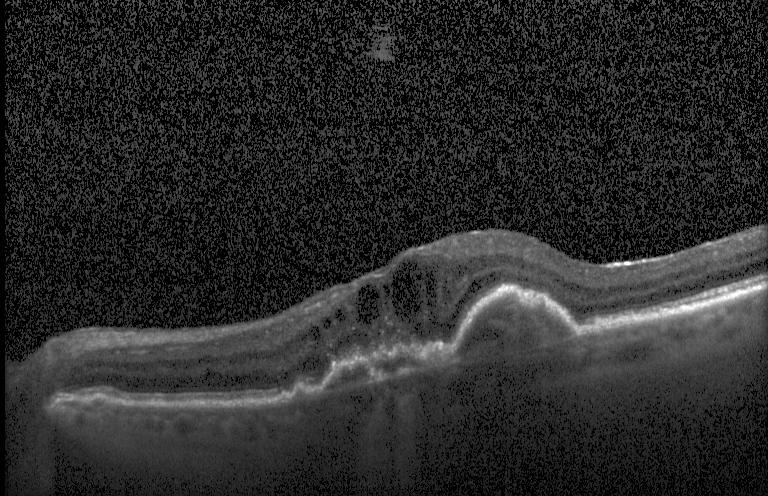 Optical coherence tomography scan
Finding: a choroidal neovascular membrane.